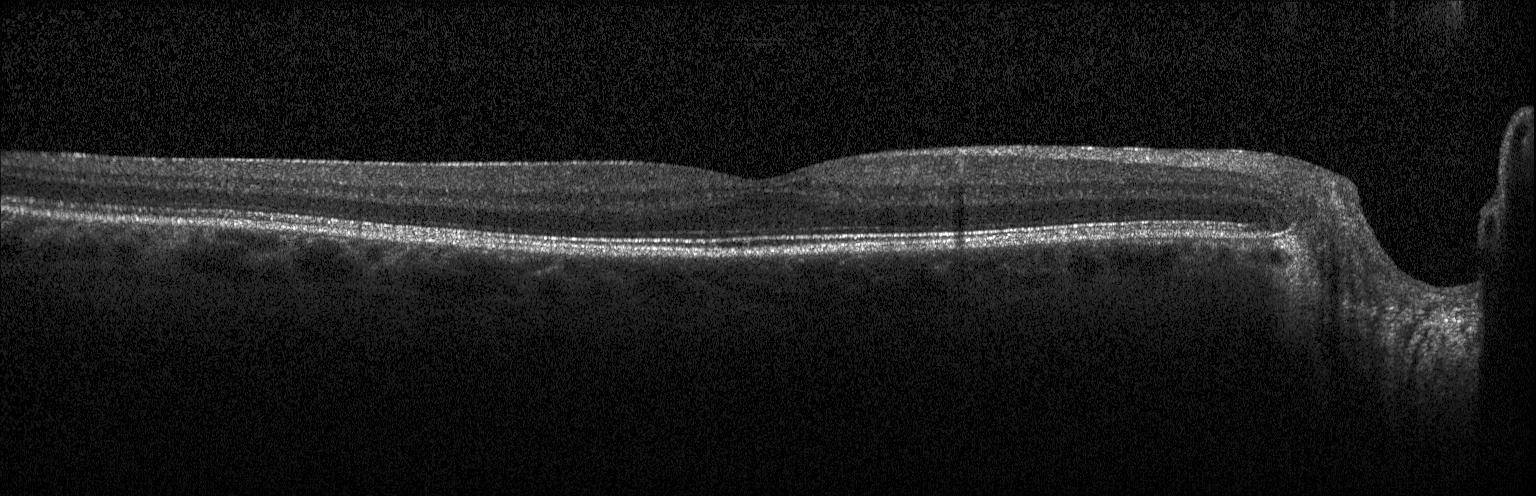 Macular scan. Retinal OCT B-scan. Acquired on a Heidelberg Spectralis. Spectral-domain OCT.
Diagnosis: no evidence of choroidal neovascularization, diabetic macular edema, or drusen.